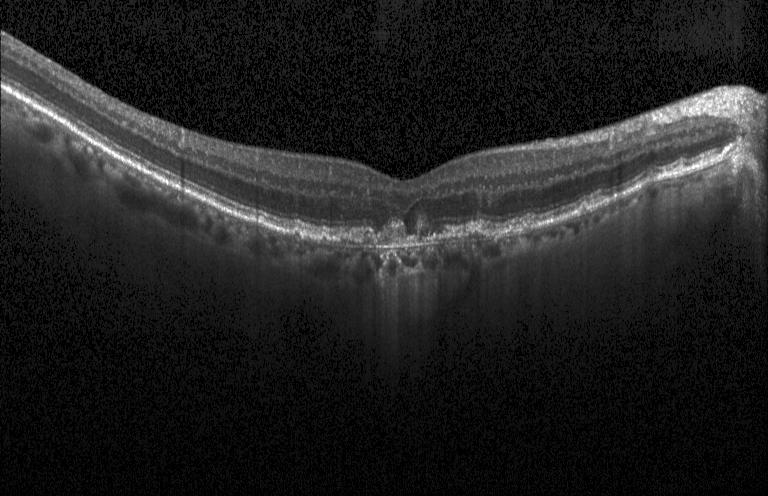 Finding: CNV.